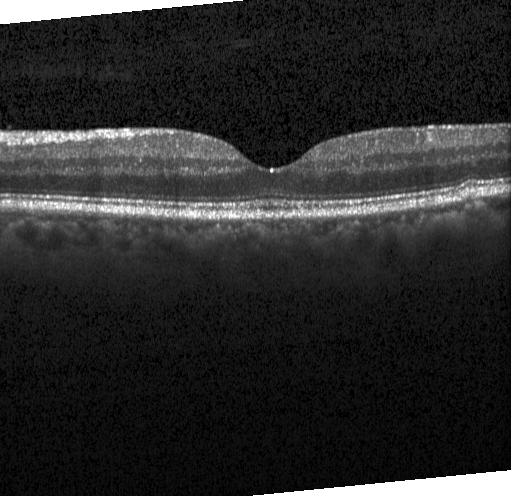 Fovea-centered, retinal OCT cross-section, acquired on a Heidelberg Spectralis. OCT finding: no choroidal neovascularization, no diabetic macular edema, and no drusen.